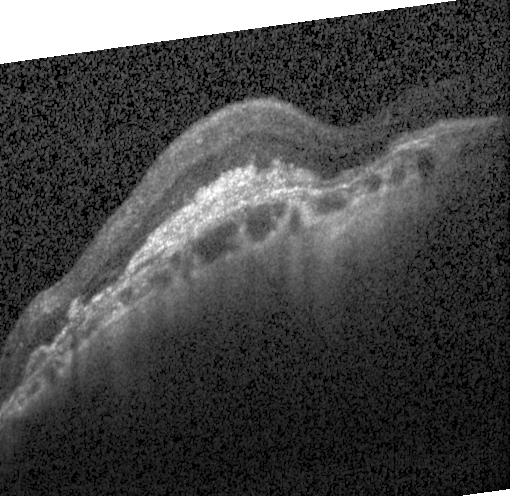
Choroidal neovascularization.